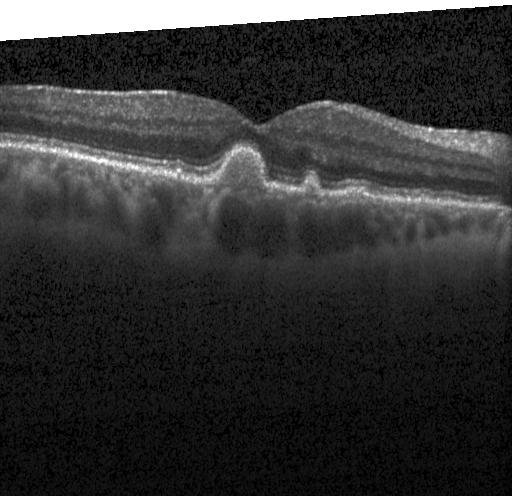

The scan shows sub-RPE drusenoid deposits.